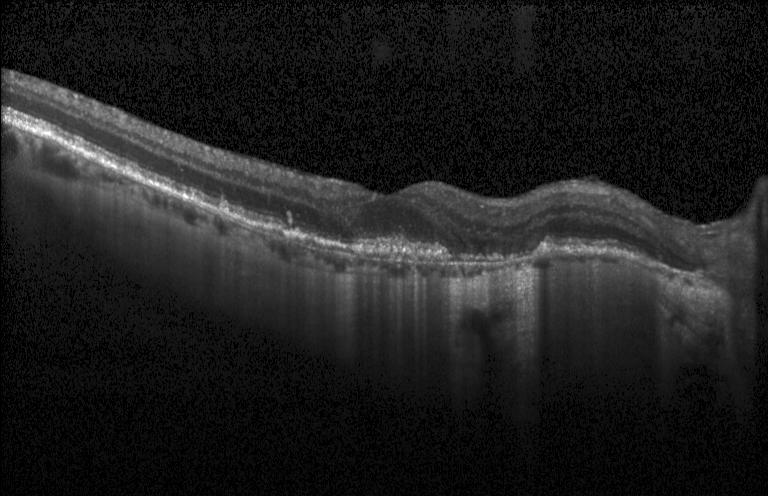
SD-OCT · Heidelberg Spectralis OCT system · OCT B-scan.
Impression: choroidal neovascularization (CNV).